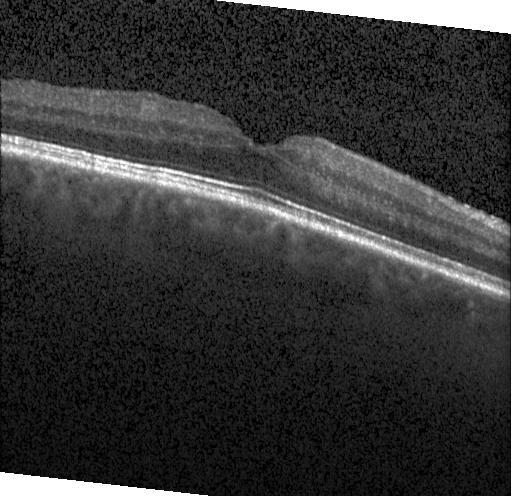

Optical coherence tomography B-scan. Fovea-centered. Acquired on a Heidelberg Spectralis
OCT finding: neither choroidal neovascularization, diabetic macular edema, nor drusen.